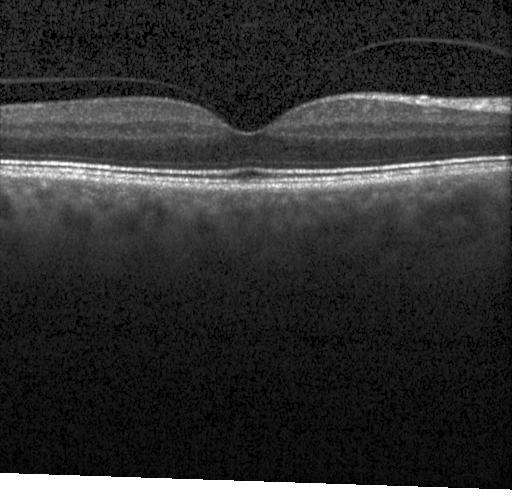
OCT line scan; SD-OCT.
Macular OCT: no choroidal neovascularization, no diabetic macular edema, and no drusen.